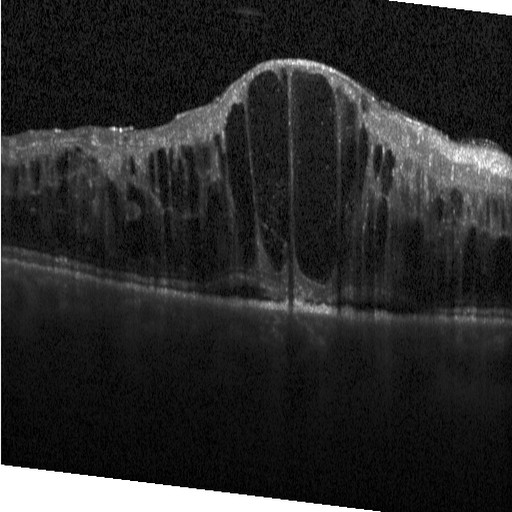

Heidelberg Spectralis. Retinal OCT B-scan. Macular OCT: diabetic macular edema.